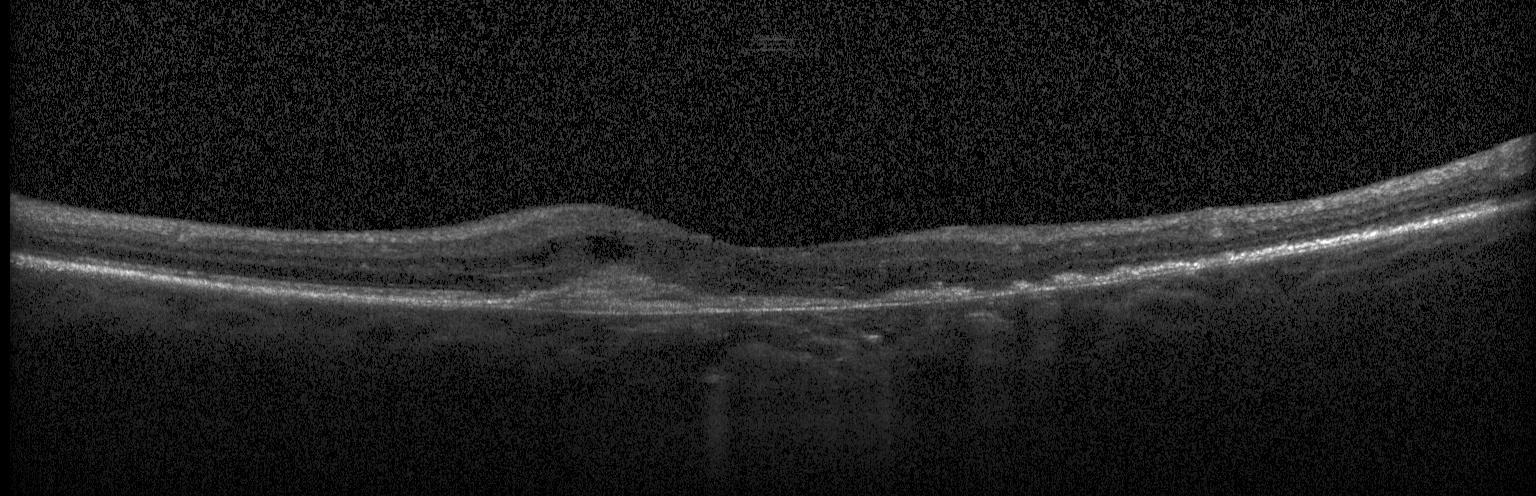
Spectral-domain OCT; retinal OCT cross-section; through the macula
A choroidal neovascular membrane.